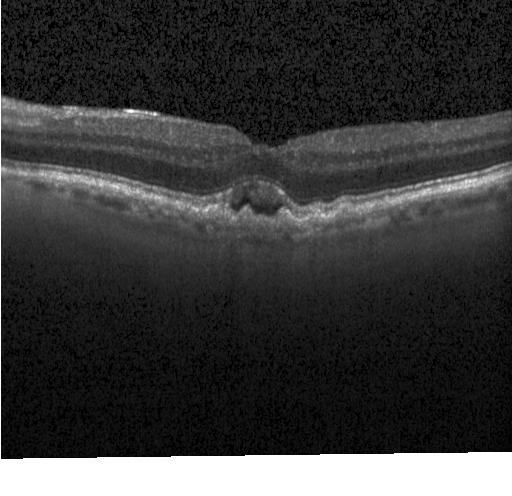
OCT B-scan — The scan shows a choroidal neovascular membrane.